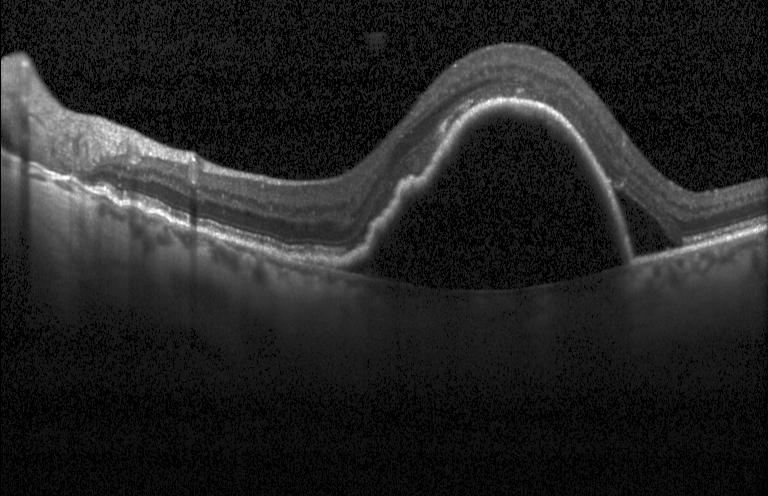
Macular OCT: choroidal neovascularization.